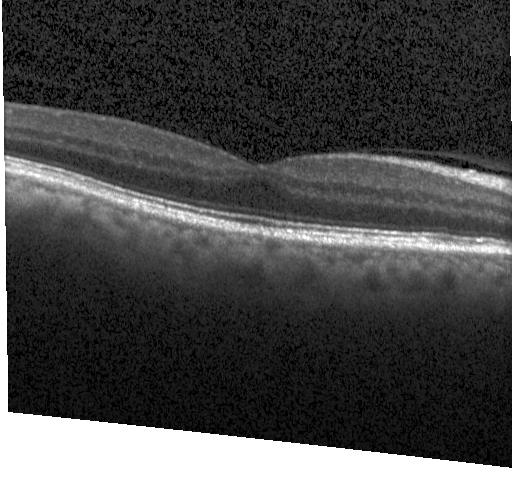

Retinal OCT B-scan · SD-OCT · horizontal scan through the fovea · Heidelberg Spectralis OCT system. Assessment: no choroidal neovascularization, no diabetic macular edema, and no drusen.